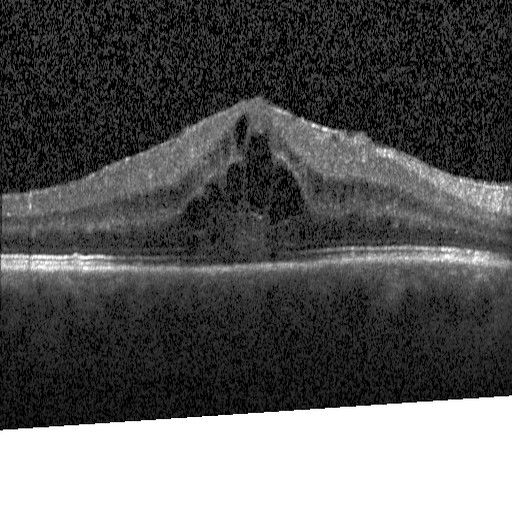 Finding: diabetic macular edema.